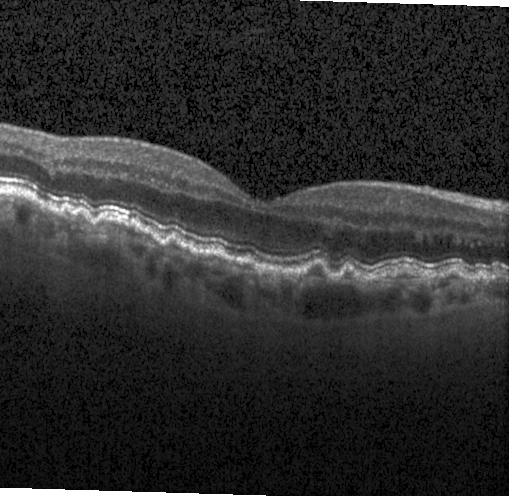

Macular scan; Heidelberg Spectralis OCT system; spectral-domain OCT; retinal OCT B-scan — OCT finding: drusen.